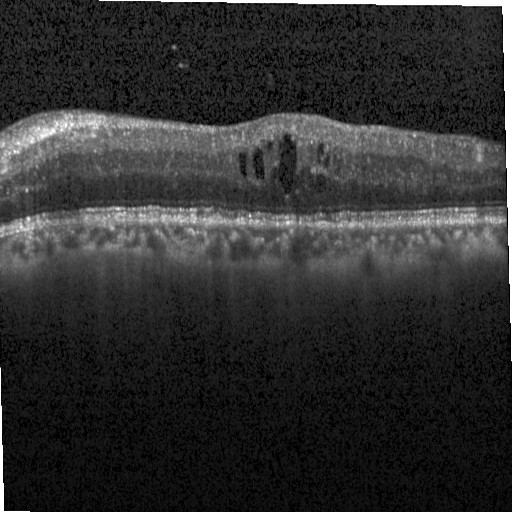 Acquired on a Heidelberg Spectralis, OCT B-scan, centered on the fovea, spectral-domain optical coherence tomography — Macular OCT: DME.